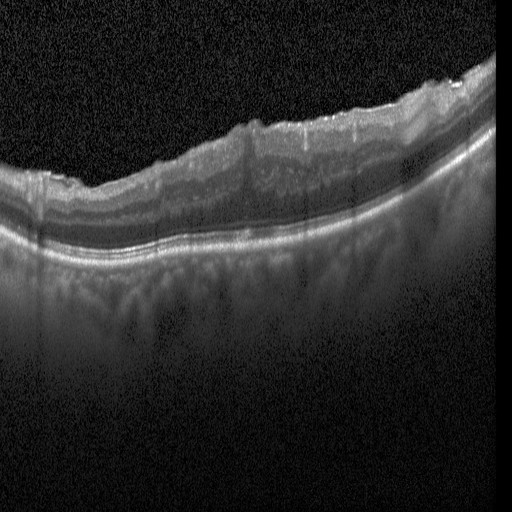
Dx: diabetic macular edema.